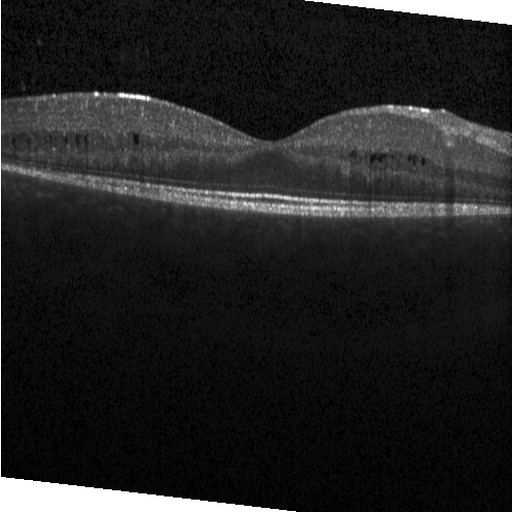

Finding: diabetic macular edema (DME).